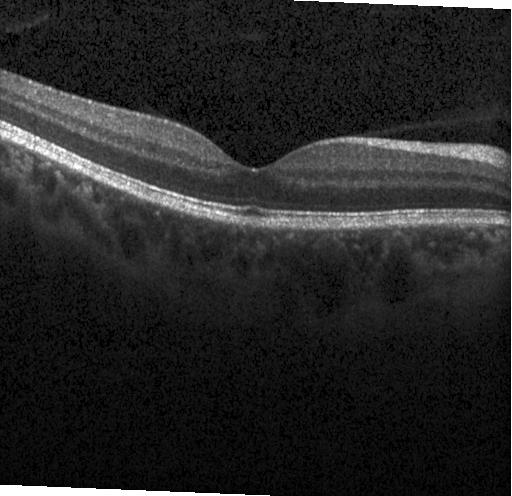
Retinal OCT cross-section showing no evidence of choroidal neovascularization, diabetic macular edema, or drusen.